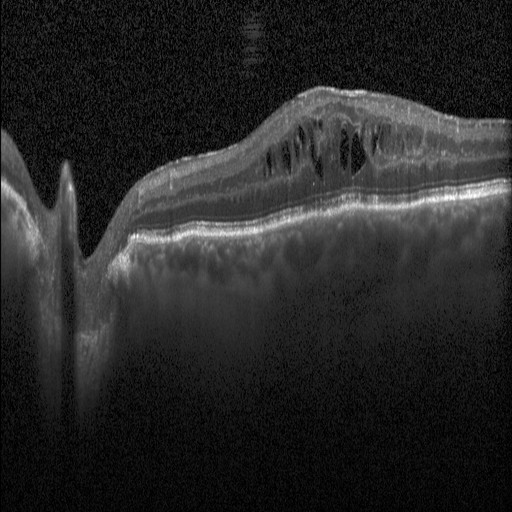

Centered on the fovea; spectral-domain OCT; Heidelberg Spectralis; OCT B-scan
Finding: diabetic macular edema (DME).